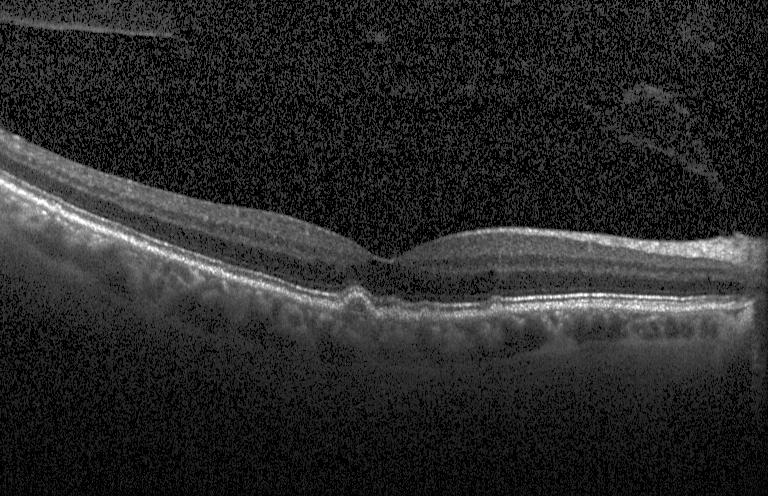

OCT line scan — Finding: drusen.